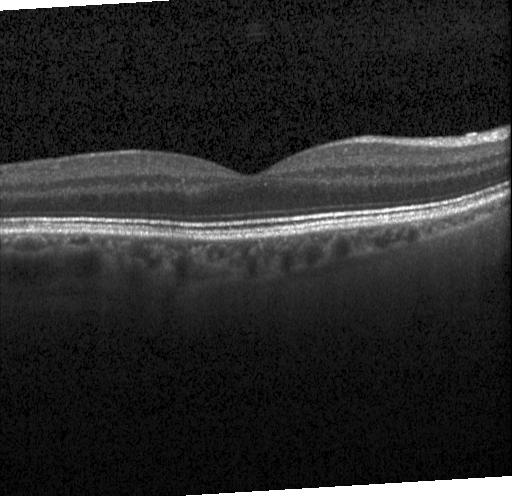
Finding: no choroidal neovascularization, diabetic macular edema, or drusen.